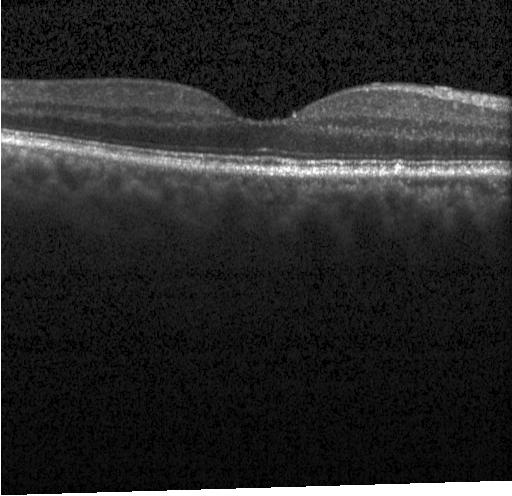
Spectral-domain optical coherence tomography, acquired on a Heidelberg Spectralis, horizontal scan through the fovea, optical coherence tomography scan — Impression: no CNV, DME, or drusen.